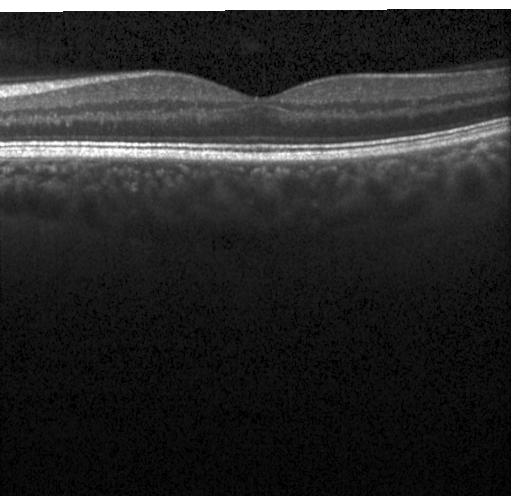
Impression: neither CNV, DME, nor drusen.